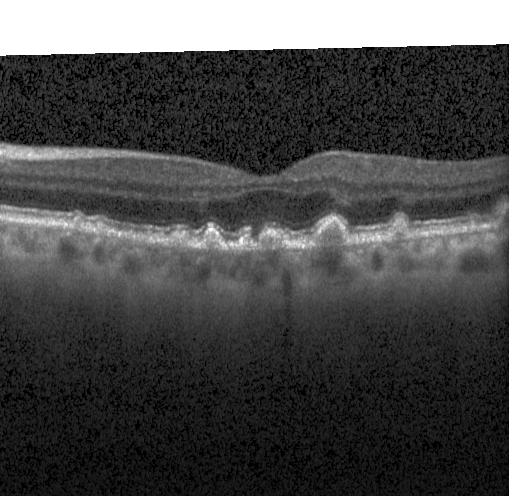
Diagnosis: multiple drusen.